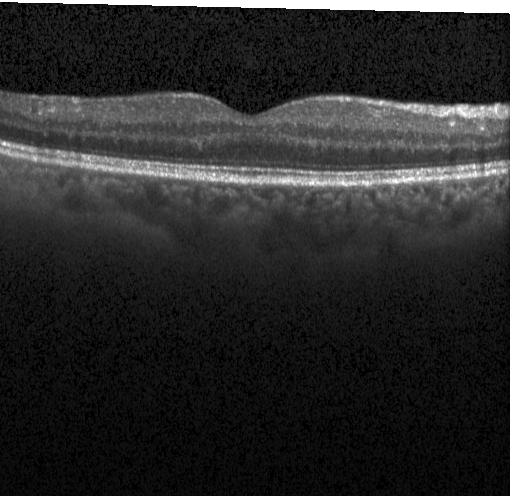 This B-scan demonstrates neither choroidal neovascularization, diabetic macular edema, nor drusen.